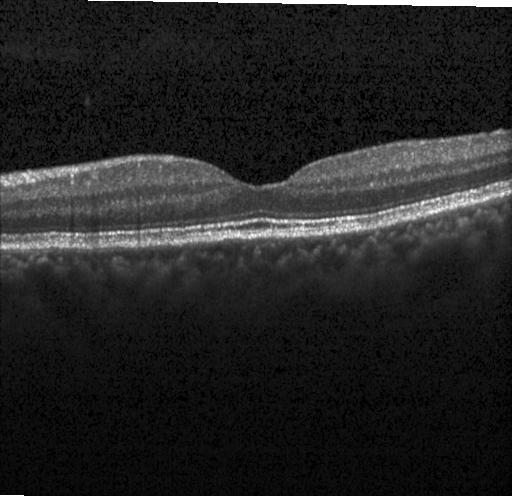

OCT line scan · macular scan
Diagnosis: no choroidal neovascularization, diabetic macular edema, or drusen.